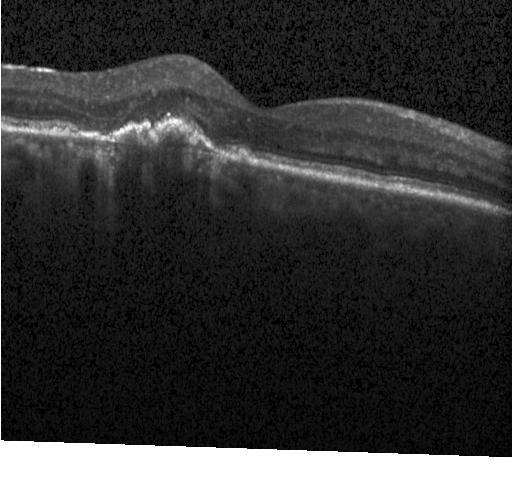

Fovea-centered. Optical coherence tomography B-scan. Spectral-domain optical coherence tomography. Heidelberg Spectralis.
Macular OCT: choroidal neovascularization.